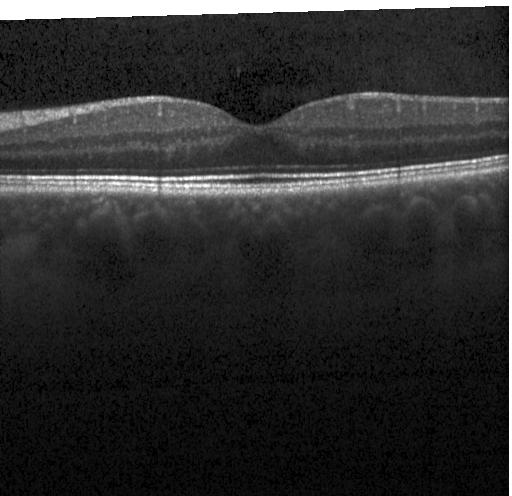 Finding: no choroidal neovascularization, no diabetic macular edema, and no drusen.